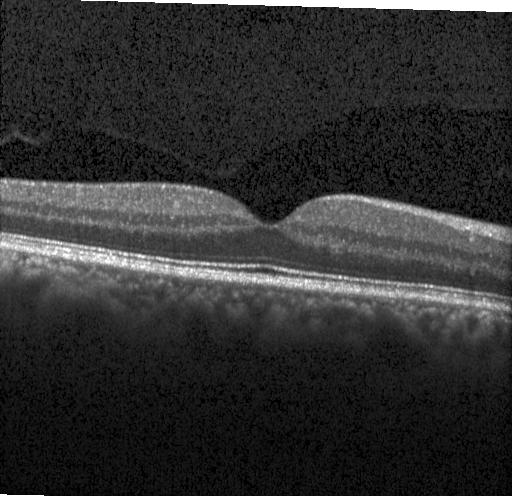

Diagnosis: no choroidal neovascularization, diabetic macular edema, or drusen.